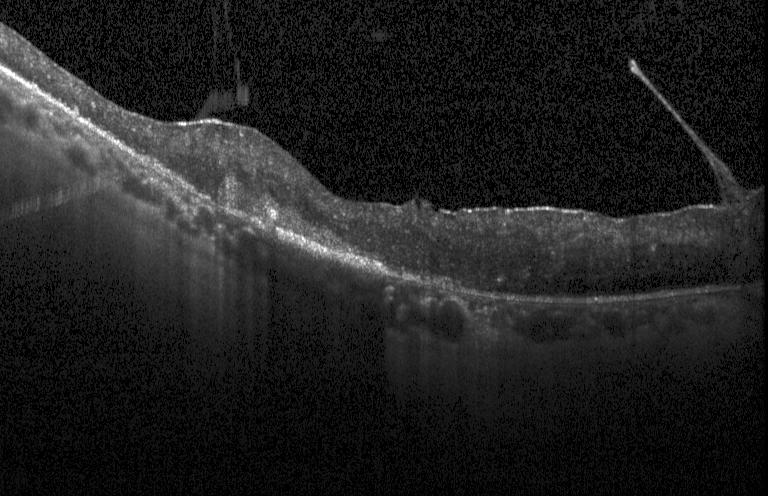

OCT B-scan showing a choroidal neovascular membrane.